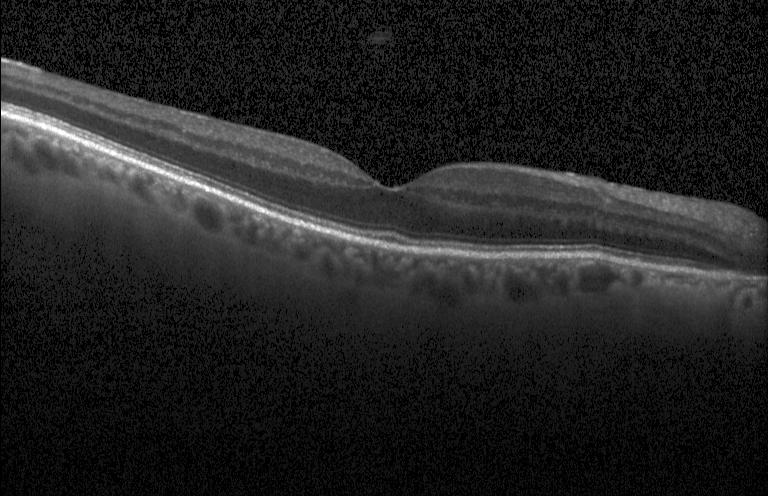
Instrument: Heidelberg Spectralis · centered on the fovea · optical coherence tomography B-scan.
Dx: neither CNV, DME, nor drusen.